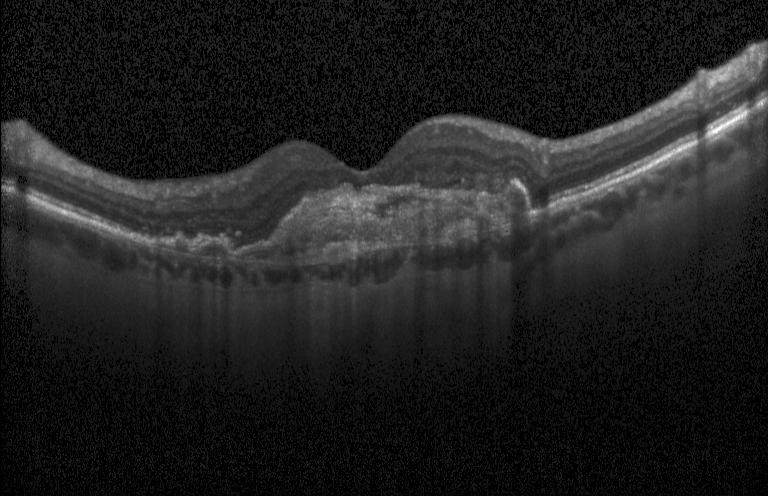

Retinal OCT cross-section — Finding: a choroidal neovascular membrane.